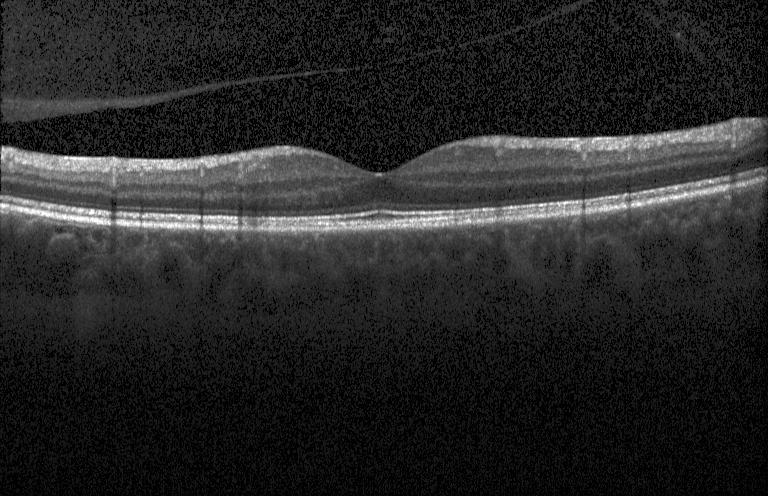

Retinal OCT cross-section showing no choroidal neovascularization, diabetic macular edema, or drusen.